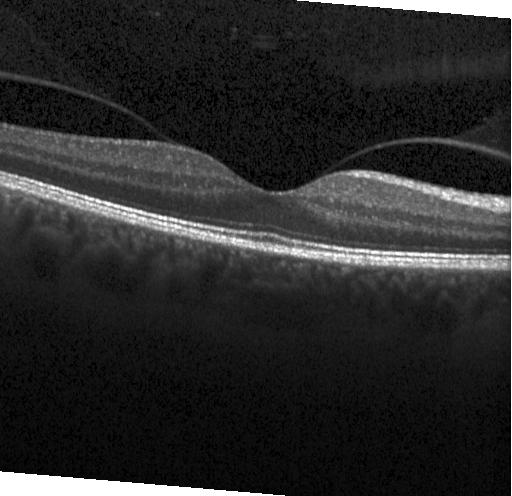

Optical coherence tomography B-scan.
Impression: no evidence of choroidal neovascularization, diabetic macular edema, or drusen.